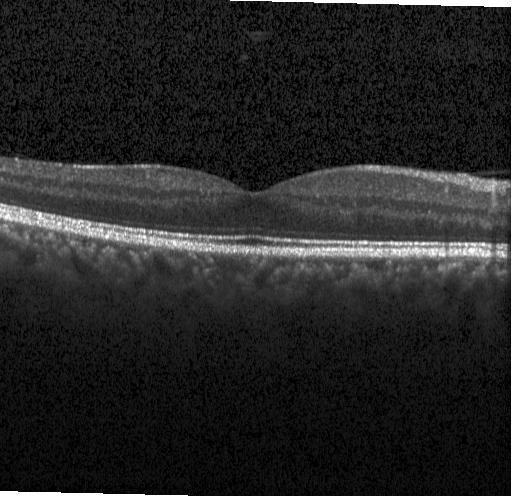
Diagnosis: no CNV, DME, or drusen.